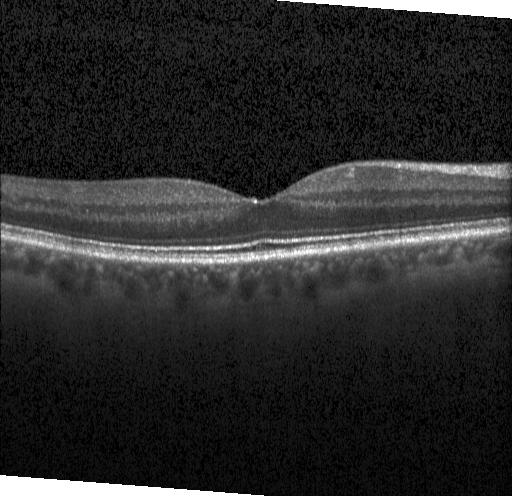 Retinal OCT B-scan; SD-OCT — Finding: no choroidal neovascularization, diabetic macular edema, or drusen.